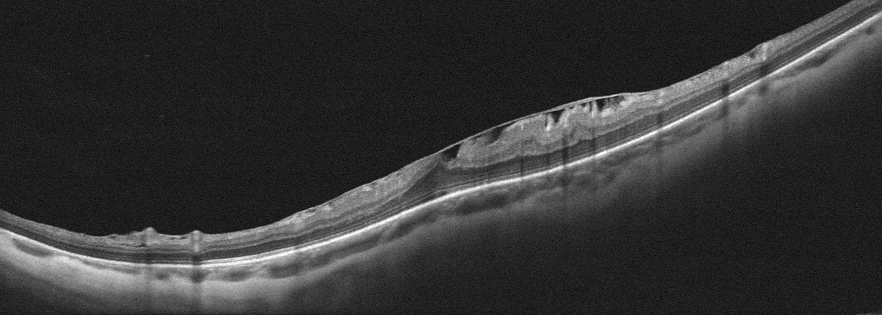
OCT line scan.
Finding: epiretinal membrane (ERM).